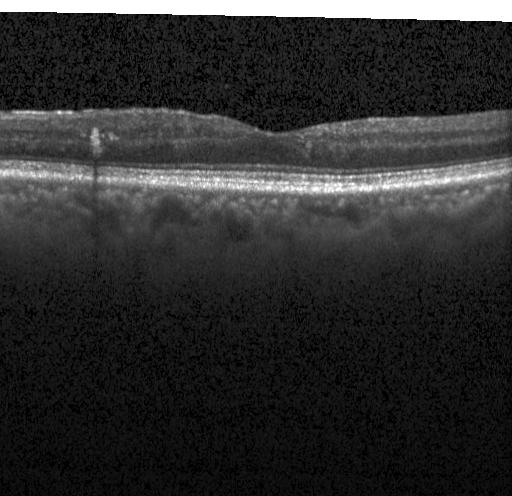
This B-scan demonstrates no CNV, DME, or drusen.